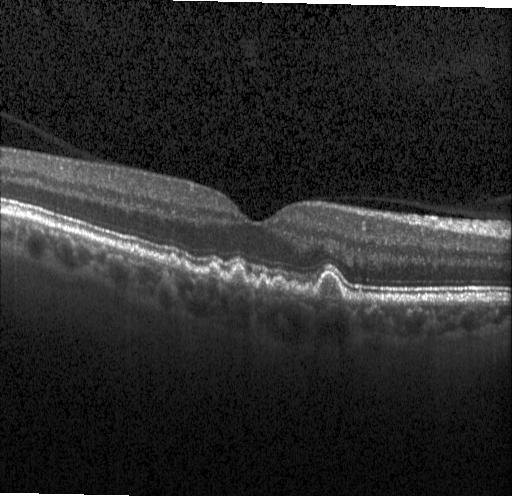
Instrument: Heidelberg Spectralis. OCT line scan. Macular scan. Spectral-domain OCT
Diagnosis: multiple drusen.